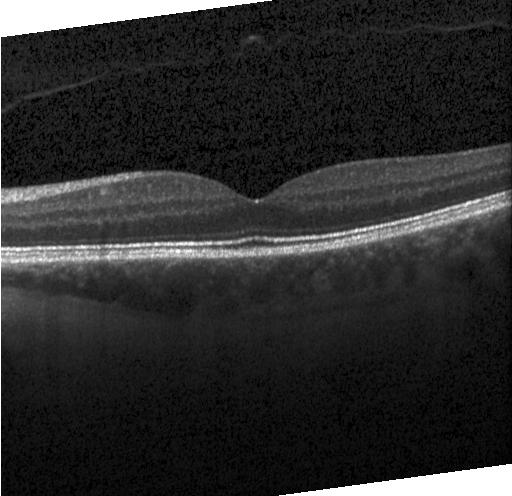
SD-OCT; retinal OCT cross-section; acquired on a Heidelberg Spectralis; centered on the fovea. Assessment: neither choroidal neovascularization, diabetic macular edema, nor drusen.